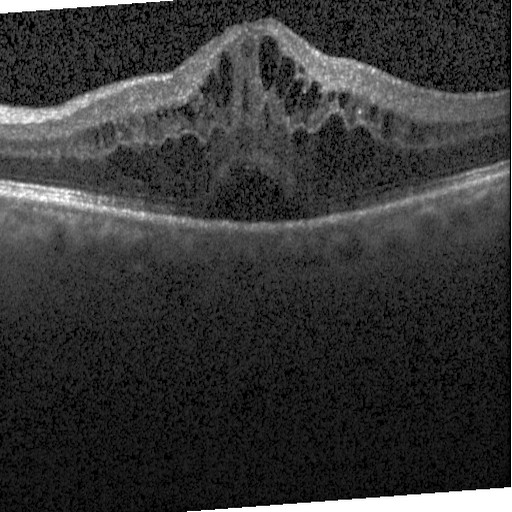

OCT line scan
Impression: diabetic macular edema.